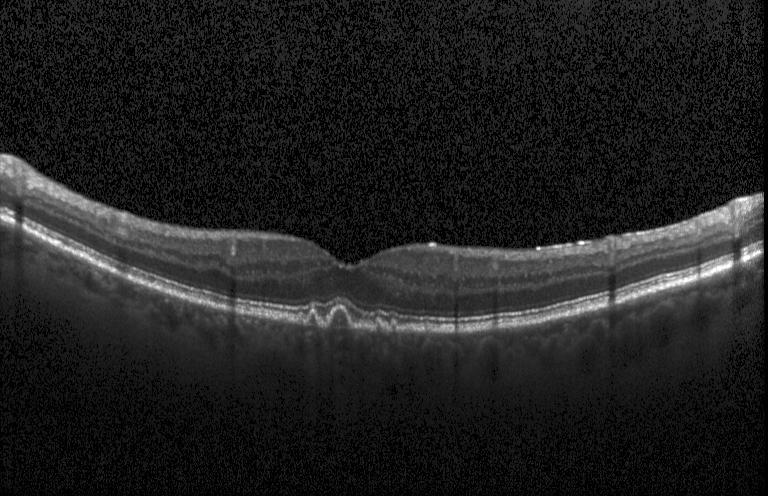

Spectral-domain optical coherence tomography, instrument: Heidelberg Spectralis, optical coherence tomography B-scan
Assessment: multiple drusen.